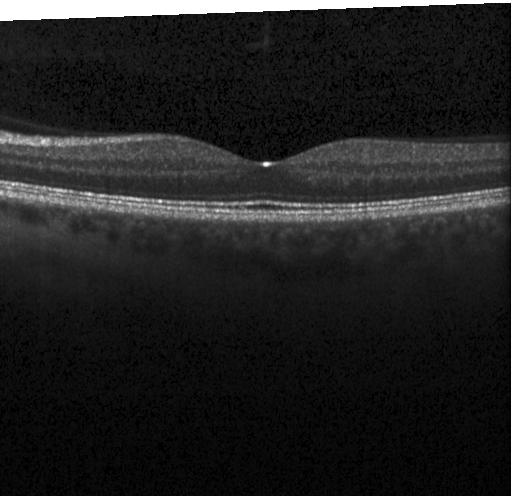

OCT B-scan, SD-OCT, instrument: Heidelberg Spectralis, horizontal scan through the fovea. OCT finding: no choroidal neovascularization, diabetic macular edema, or drusen.